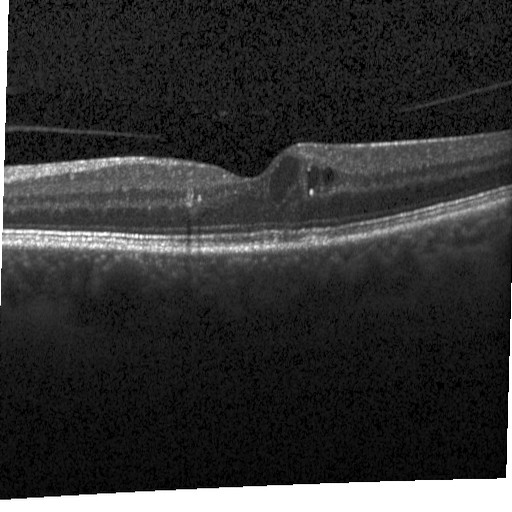

Heidelberg Spectralis · SD-OCT · OCT line scan · horizontal scan through the fovea — Diabetic macular edema.